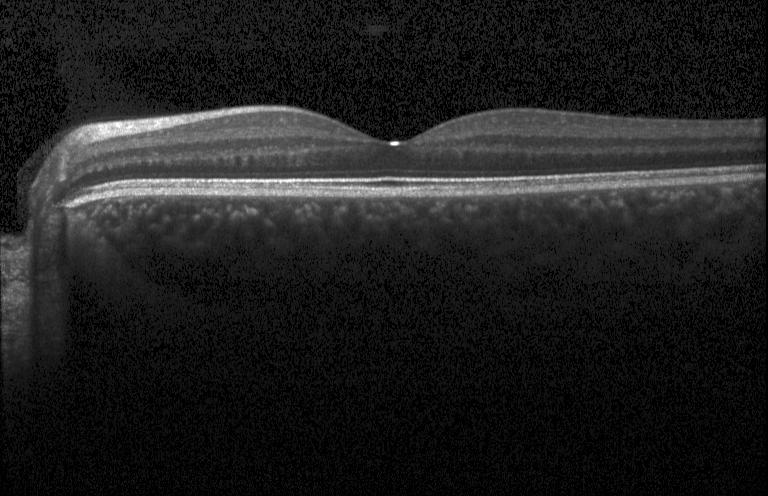

Retinal OCT cross-section
Dx: no evidence of choroidal neovascularization, diabetic macular edema, or drusen.